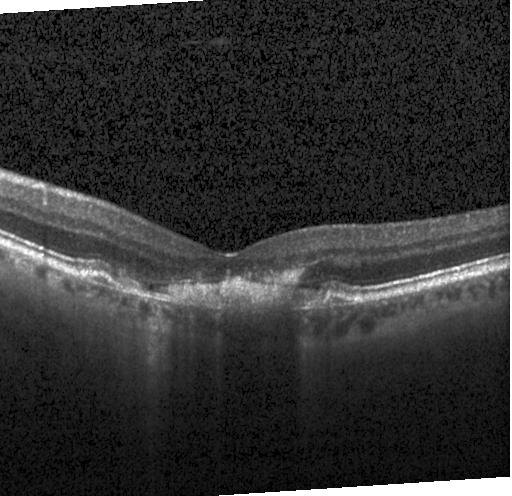
Impression: choroidal neovascularization (CNV).